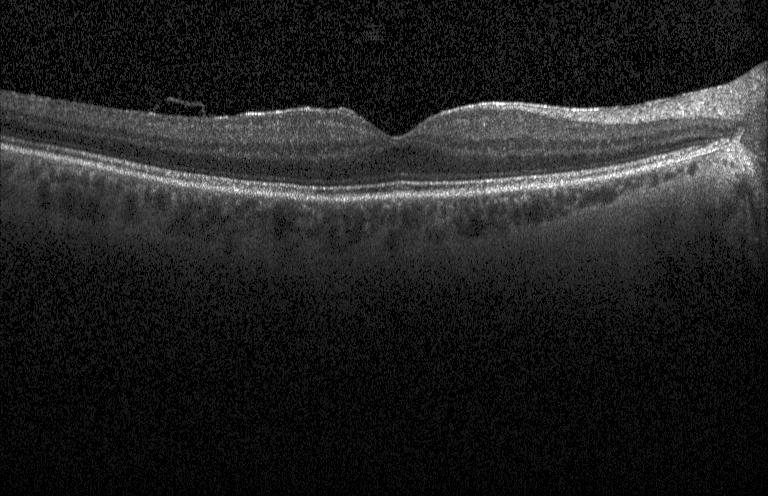 Acquired on a Heidelberg Spectralis. OCT B-scan. This B-scan demonstrates neither CNV, DME, nor drusen.